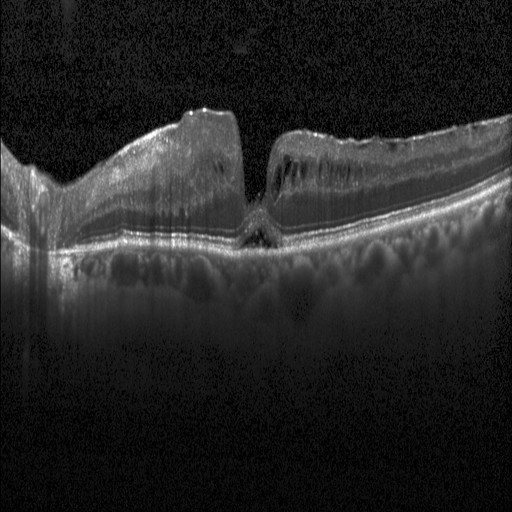
Finding: diabetic macular edema (DME).